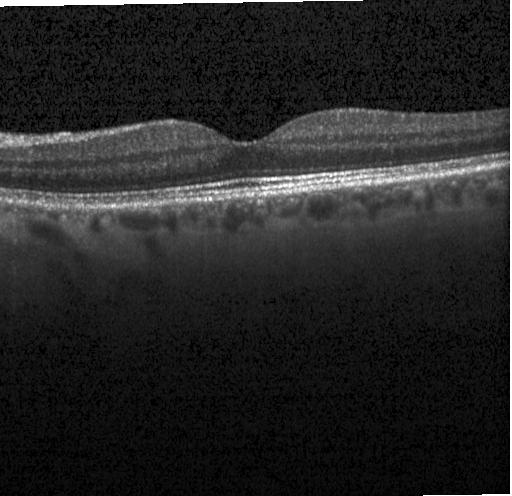

OCT line scan. Diagnosis: neither choroidal neovascularization, diabetic macular edema, nor drusen.